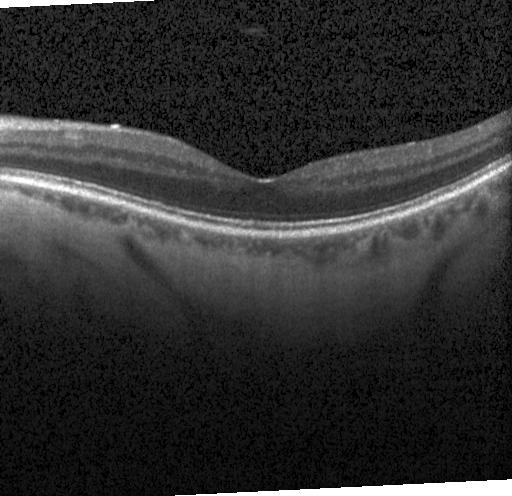
OCT B-scan.
This B-scan demonstrates no evidence of choroidal neovascularization, diabetic macular edema, or drusen.